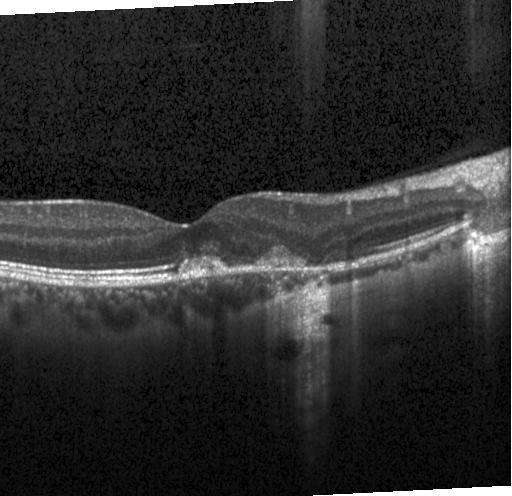
Macular OCT demonstrating choroidal neovascularization (CNV).